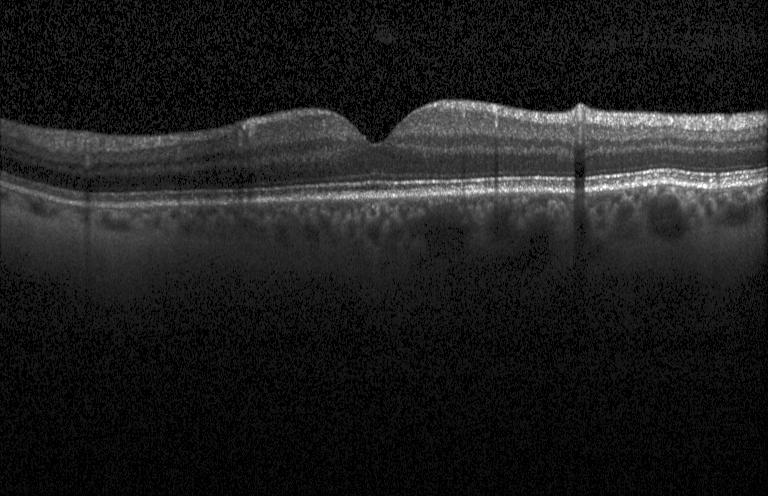

Assessment: no evidence of CNV, DME, or drusen.